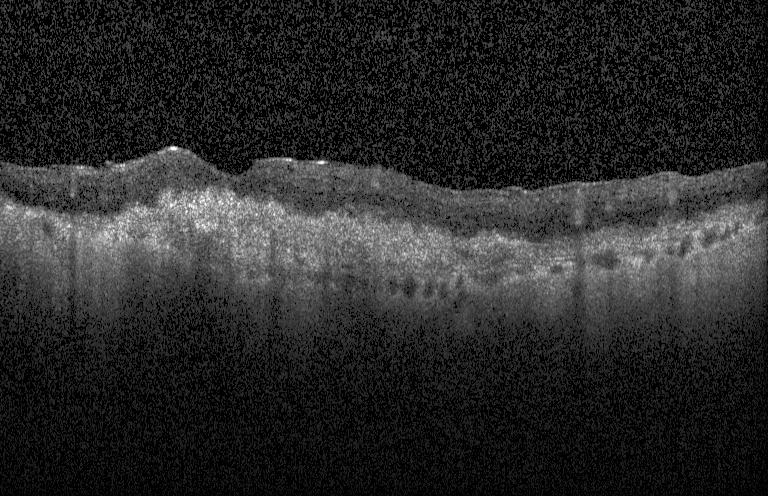 Impression: a choroidal neovascular membrane.